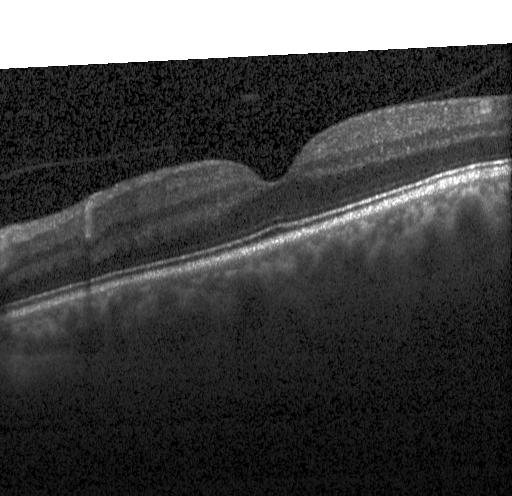

Finding: no choroidal neovascularization, diabetic macular edema, or drusen.